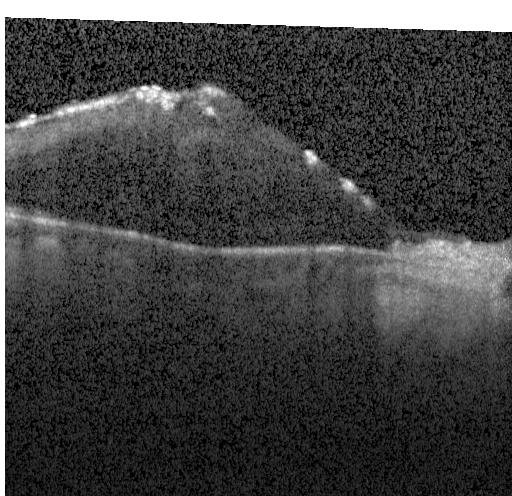 Impression: DME.